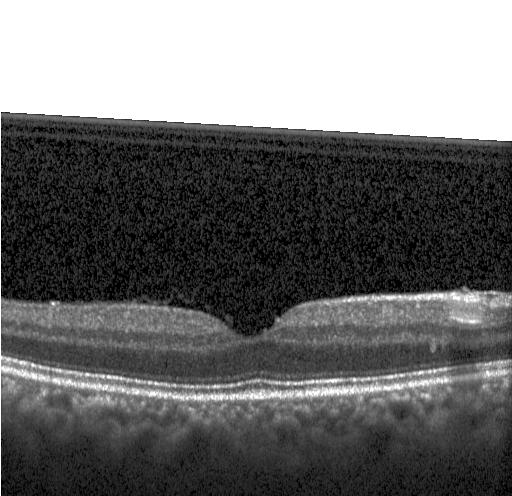 Acquired on a Heidelberg Spectralis, optical coherence tomography B-scan.
The scan shows neither choroidal neovascularization, diabetic macular edema, nor drusen.